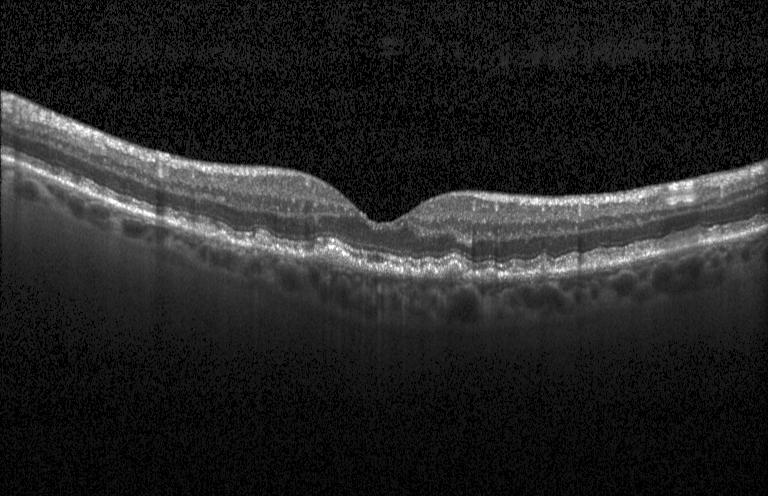

Optical coherence tomography B-scan; acquired on a Heidelberg Spectralis; through the macula; spectral-domain OCT. OCT finding: multiple drusen.